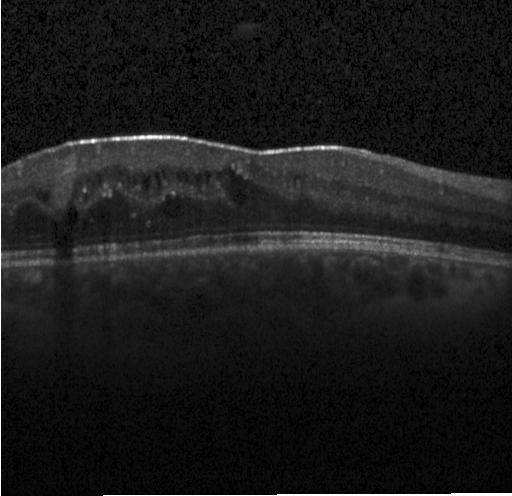

Centered on the fovea, optical coherence tomography B-scan, spectral-domain optical coherence tomography — Assessment: DME.